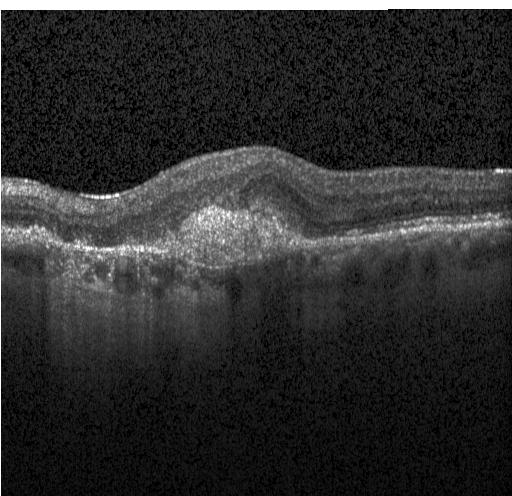
Acquired on a Heidelberg Spectralis · optical coherence tomography B-scan — Finding: CNV.